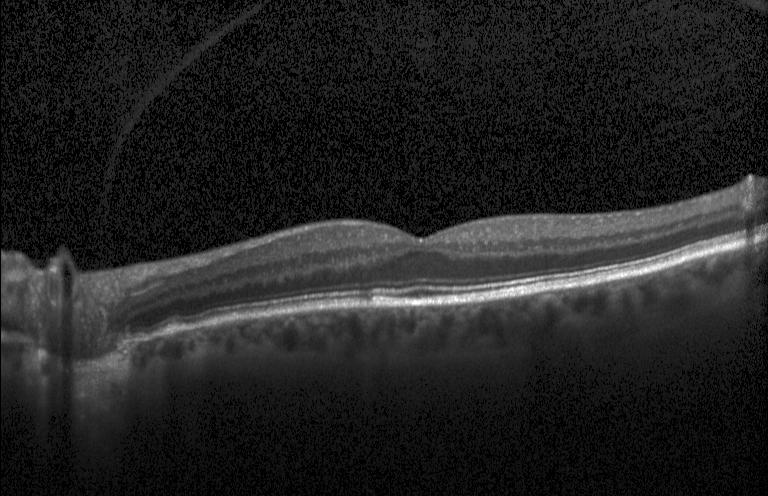
Retinal OCT B-scan; spectral-domain OCT; instrument: Heidelberg Spectralis — Finding: no evidence of choroidal neovascularization, diabetic macular edema, or drusen.